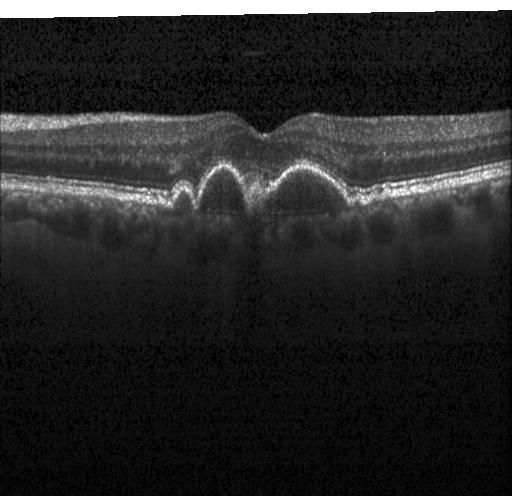
Heidelberg Spectralis OCT system · optical coherence tomography B-scan. A choroidal neovascular membrane.